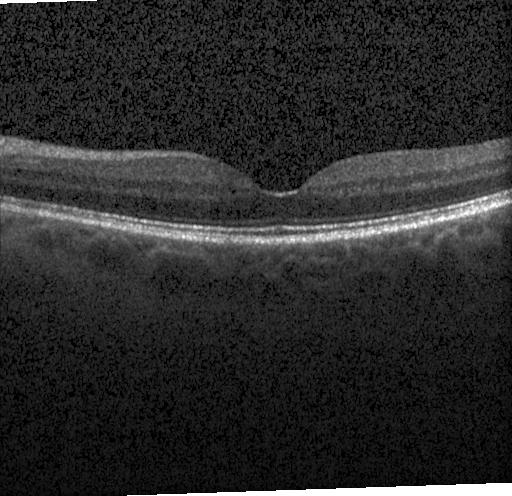
OCT B-scan · SD-OCT. Finding: no choroidal neovascularization, no diabetic macular edema, and no drusen.